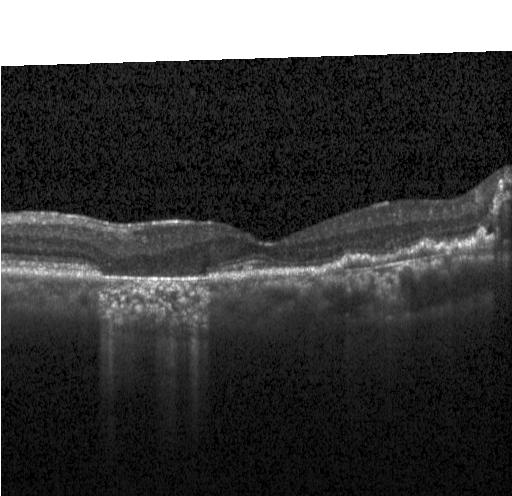

Impression: choroidal neovascularization (CNV).